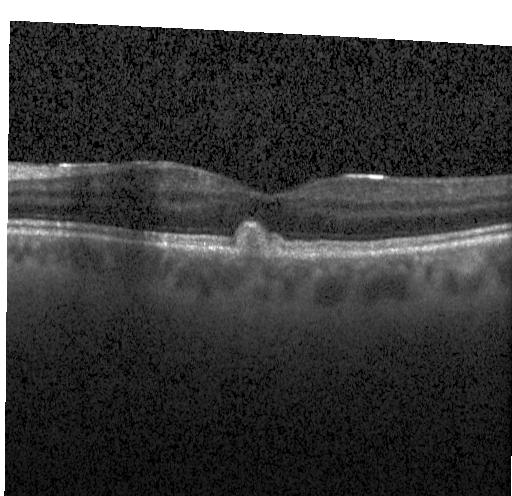

Macular scan. Optical coherence tomography B-scan — Sub-RPE drusenoid deposits.